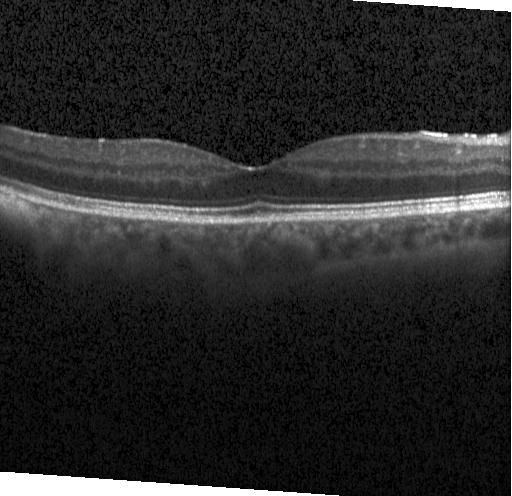

OCT line scan. The scan shows no evidence of choroidal neovascularization, diabetic macular edema, or drusen.